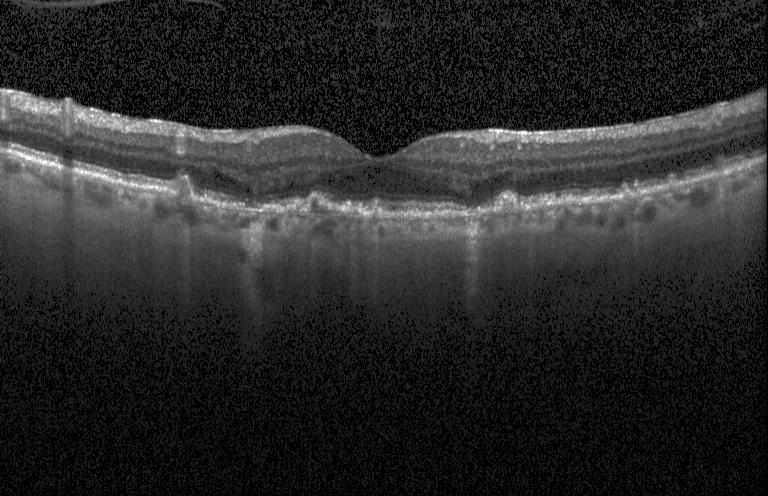
Finding: drusen.